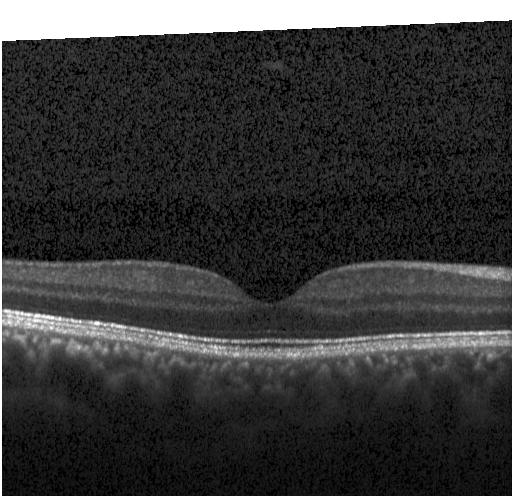

Retinal OCT cross-section. The scan shows no CNV, DME, or drusen.